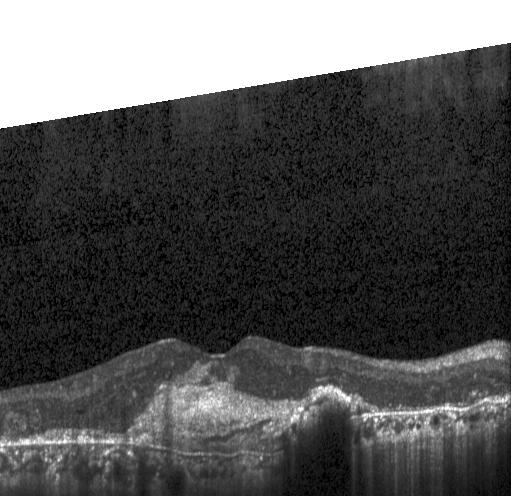

Dx: a choroidal neovascular membrane.